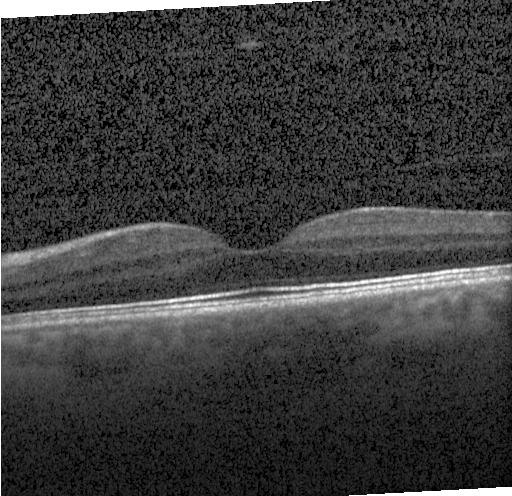 OCT B-scan
The scan shows no choroidal neovascularization, no diabetic macular edema, and no drusen.